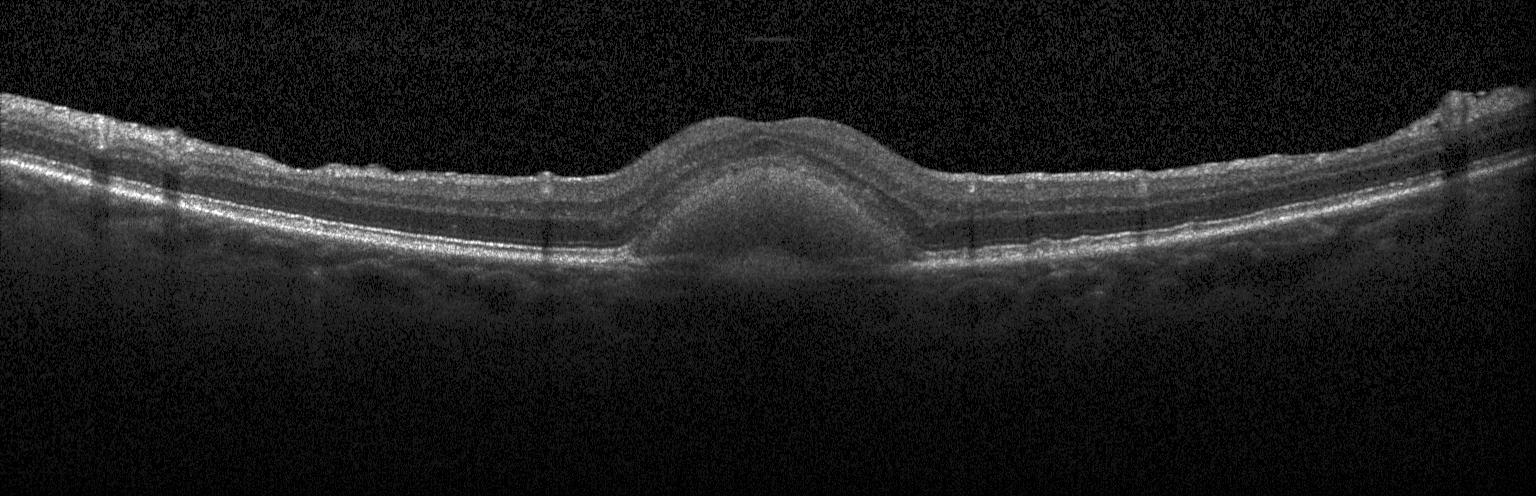
Centered on the fovea, SD-OCT, retinal OCT B-scan
Impression: a choroidal neovascular membrane.